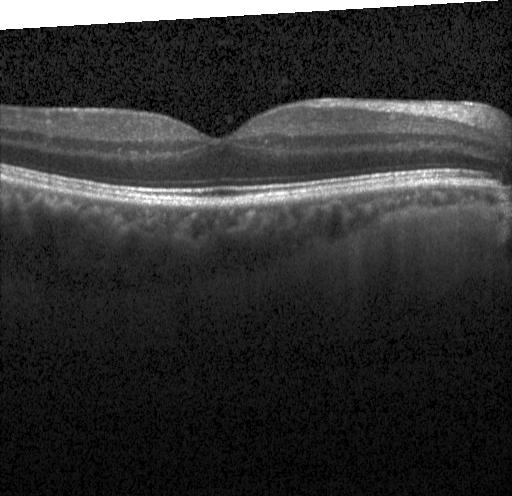 Retinal OCT cross-section showing neither choroidal neovascularization, diabetic macular edema, nor drusen.